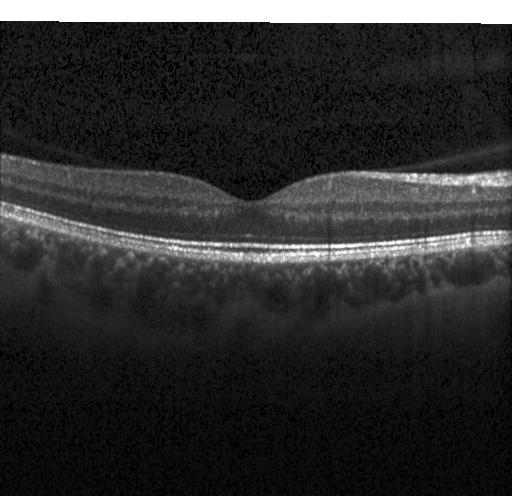 Impression: no choroidal neovascularization, no diabetic macular edema, and no drusen.